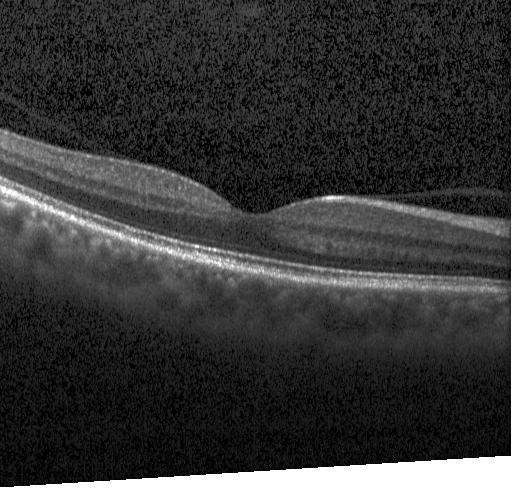
Spectral-domain optical coherence tomography, retinal OCT cross-section, instrument: Heidelberg Spectralis, fovea-centered. Macular OCT: no evidence of CNV, DME, or drusen.